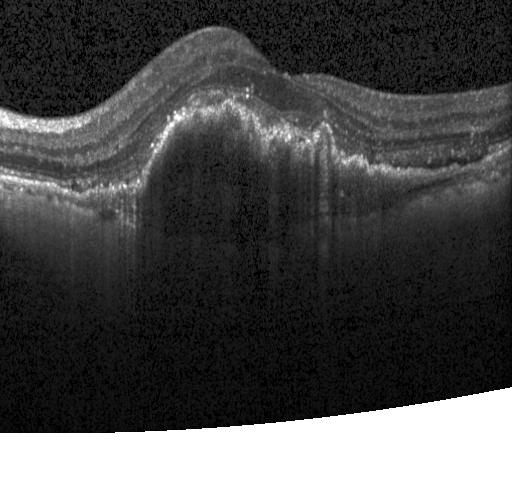 Macular OCT demonstrating choroidal neovascularization.